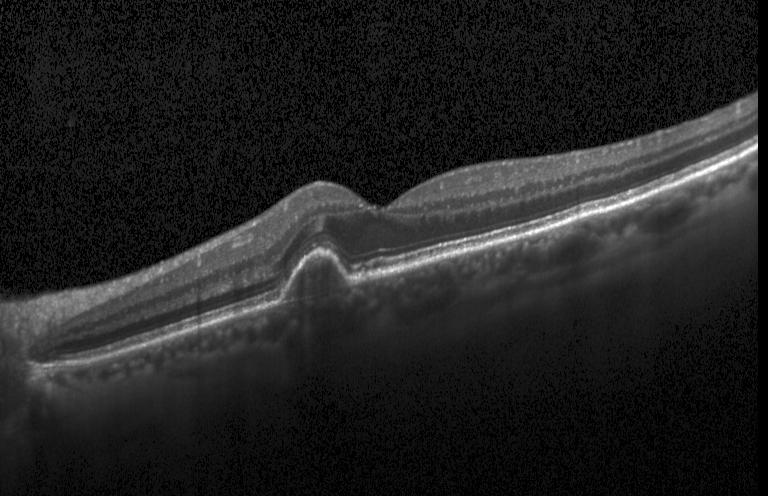
Spectral-domain OCT; instrument: Heidelberg Spectralis; optical coherence tomography B-scan; fovea-centered
Diagnosis: CNV.